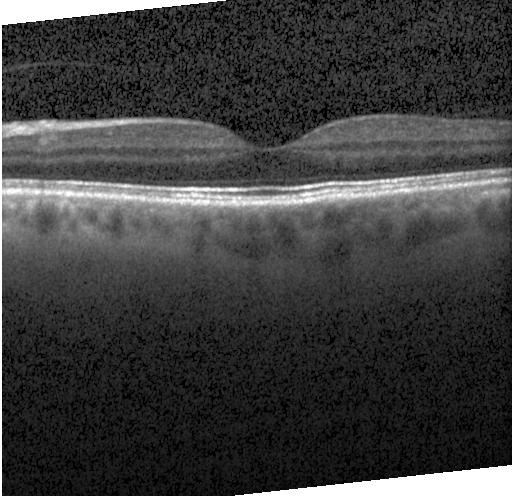 Retinal OCT cross-section
Impression: no choroidal neovascularization, diabetic macular edema, or drusen.